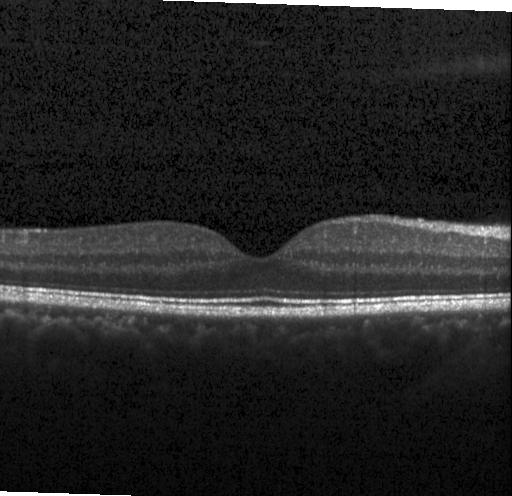

Impression: no evidence of choroidal neovascularization, diabetic macular edema, or drusen.